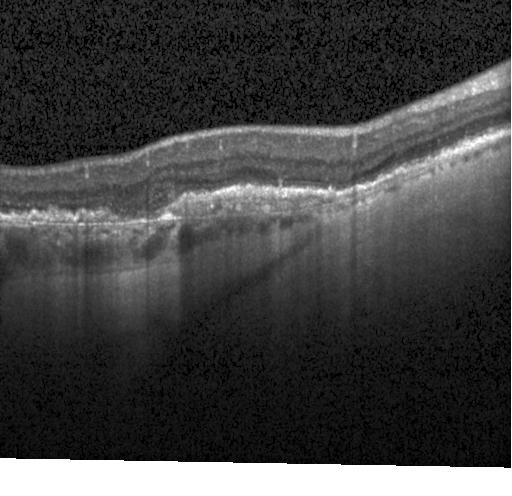 Diagnosis: CNV.